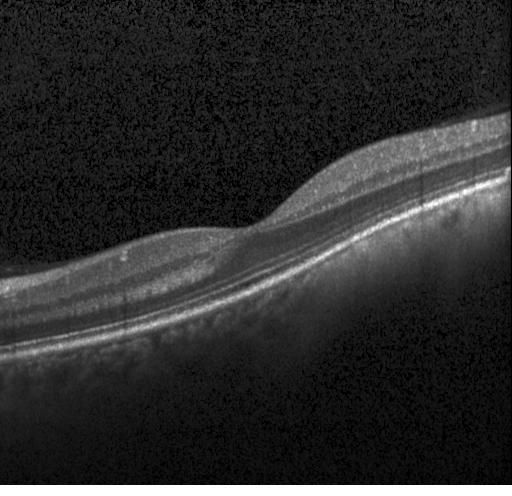 Dx: neither choroidal neovascularization, diabetic macular edema, nor drusen.